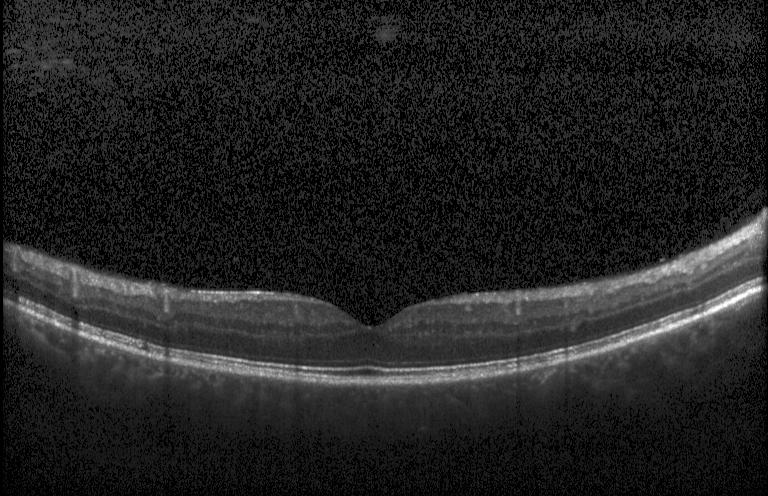
Optical coherence tomography scan
The scan shows no CNV, DME, or drusen.